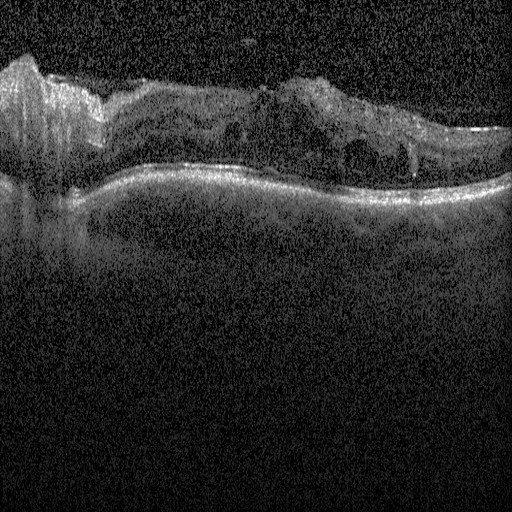
Optical coherence tomography B-scan · fovea-centered · acquired on a Heidelberg Spectralis · SD-OCT.
Diagnosis: DME.